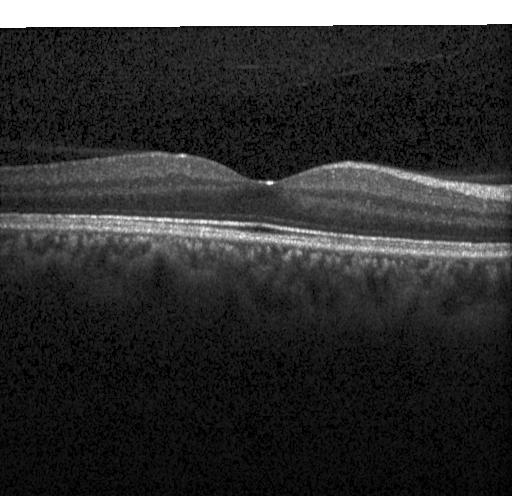

OCT finding: no choroidal neovascularization, no diabetic macular edema, and no drusen.